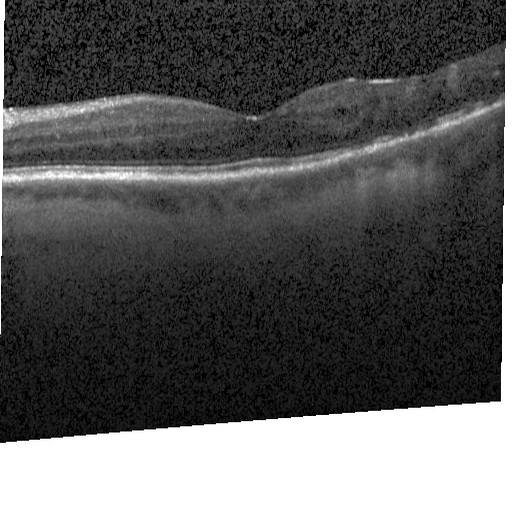 Optical coherence tomography B-scan
Finding: diabetic macular edema (DME).